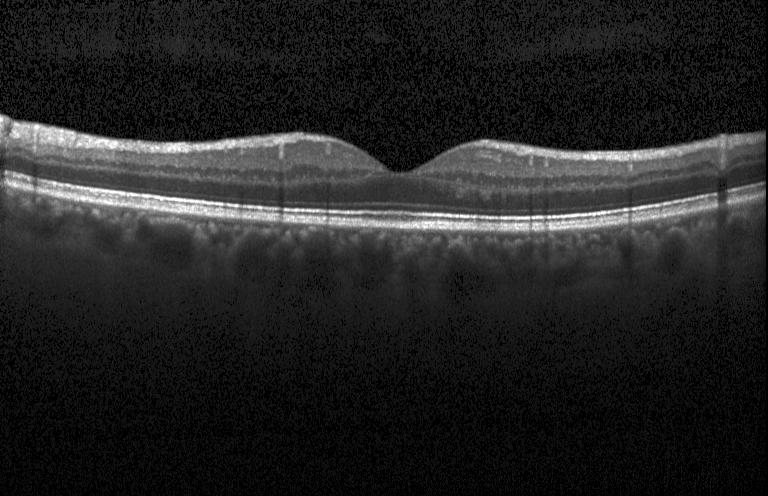 Retinal OCT cross-section; fovea-centered
No evidence of CNV, DME, or drusen.